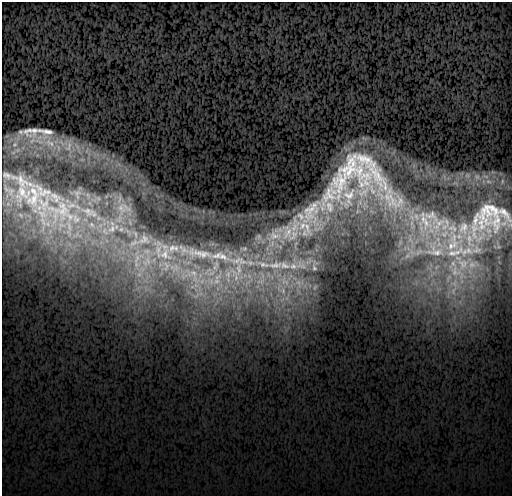
Finding: CNV.